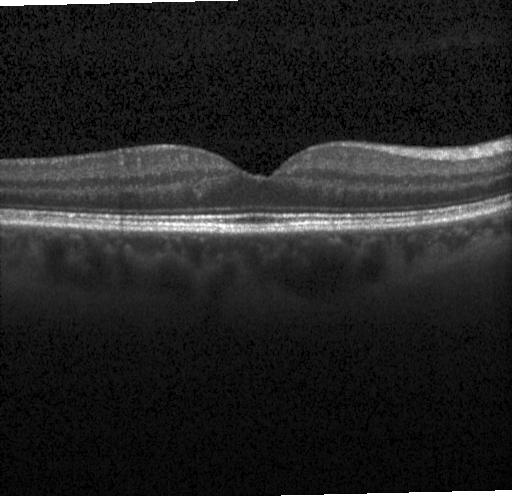 Through the macula, retinal OCT cross-section, spectral-domain OCT — Diagnosis: no evidence of choroidal neovascularization, diabetic macular edema, or drusen.